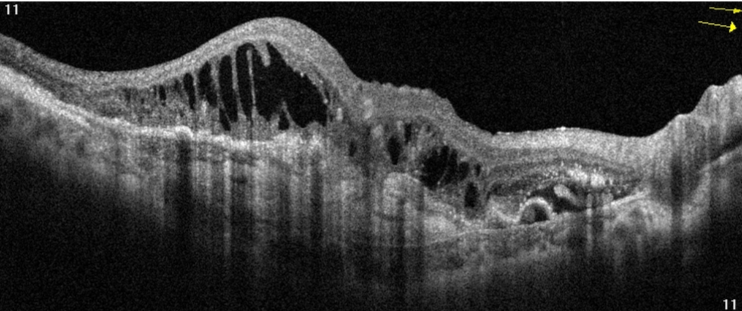
Diagnosis: AMD.